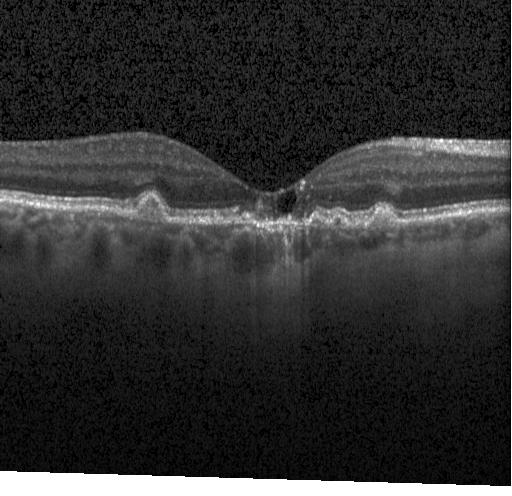 Spectral-domain OCT. Through the macula. OCT B-scan. Acquired on a Heidelberg Spectralis — OCT finding: a choroidal neovascular membrane.